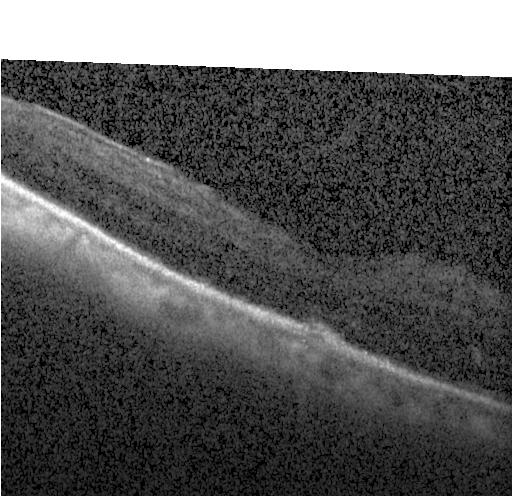

Spectral-domain OCT B-scan: CNV.